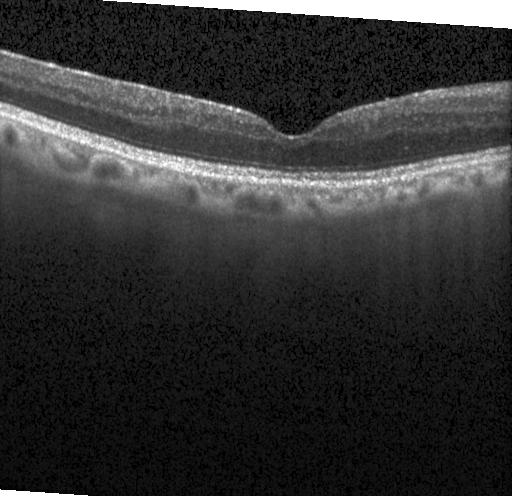 Optical coherence tomography scan. Assessment: no choroidal neovascularization, diabetic macular edema, or drusen.